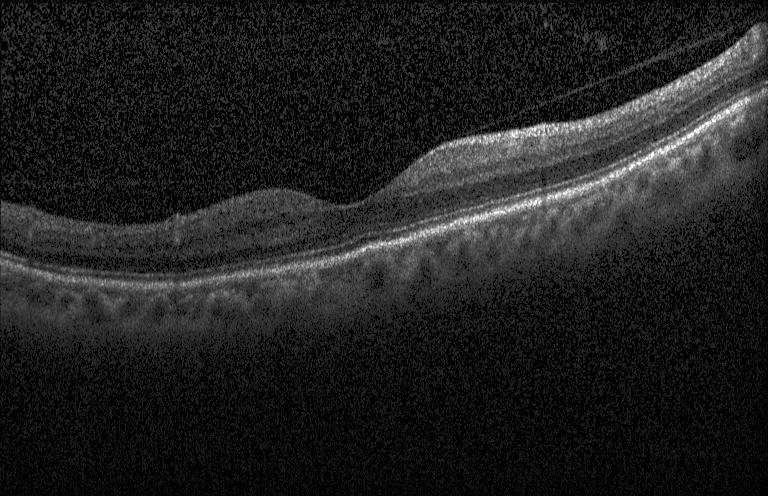

Instrument: Heidelberg Spectralis; OCT line scan.
Diagnosis: neither CNV, DME, nor drusen.